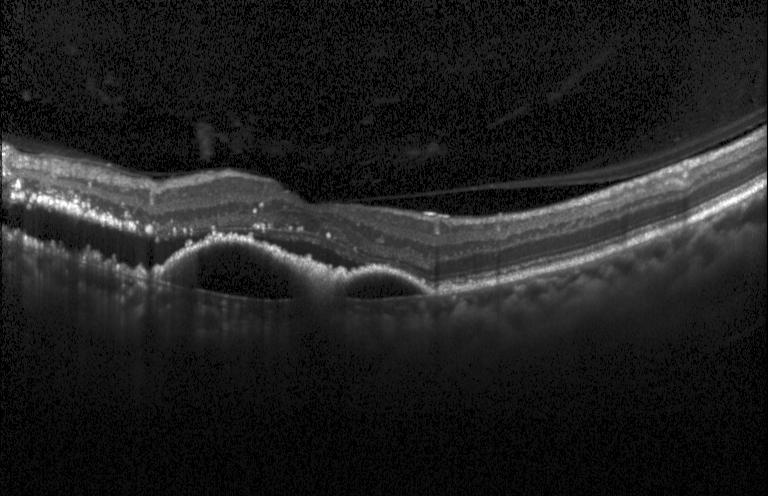 SD-OCT. Heidelberg Spectralis OCT system. Retinal OCT cross-section. OCT finding: a choroidal neovascular membrane.